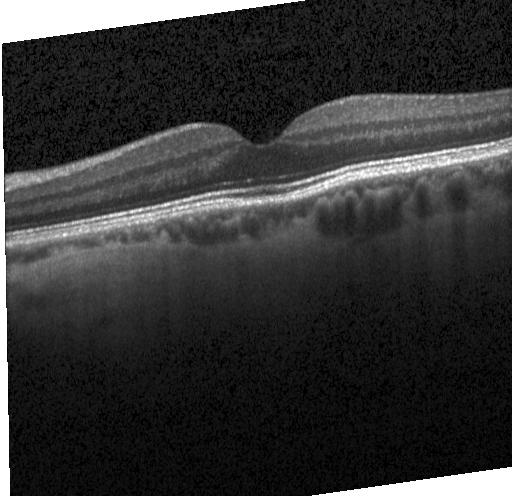 Spectral-domain OCT B-scan: no CNV, no DME, and no drusen.